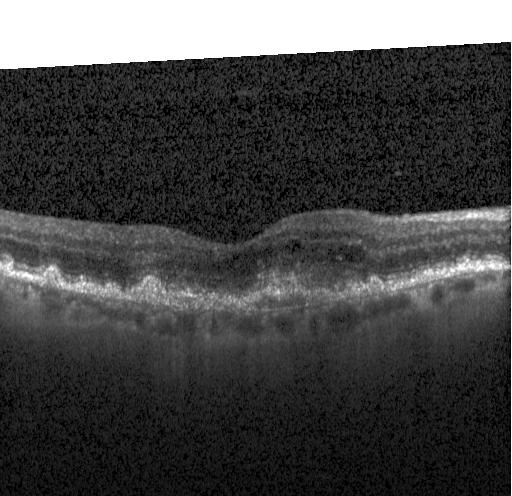

Spectral-domain optical coherence tomography. Retinal OCT B-scan. This B-scan demonstrates a choroidal neovascular membrane.